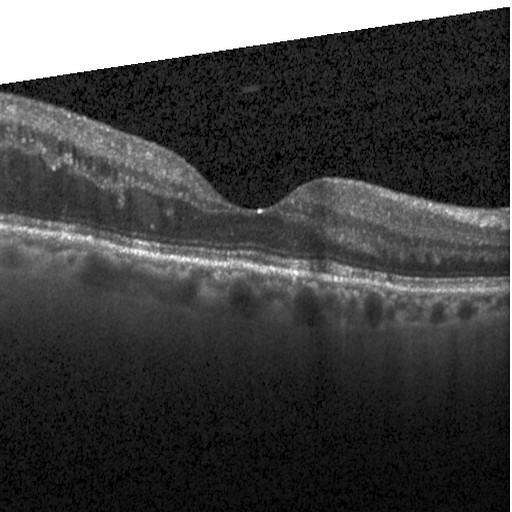
Spectral-domain OCT. Optical coherence tomography B-scan. Finding: diabetic macular edema.